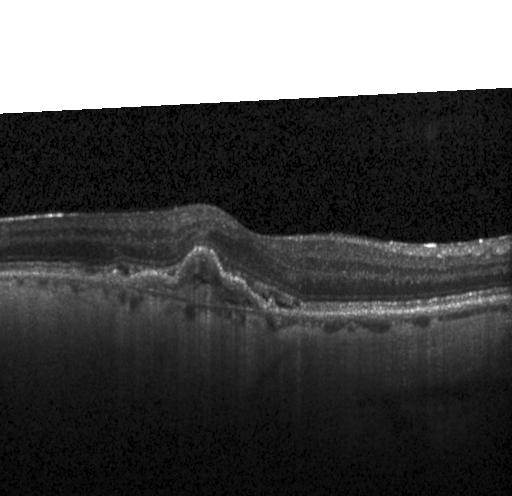
OCT B-scan. Heidelberg Spectralis — Macular OCT: a choroidal neovascular membrane.